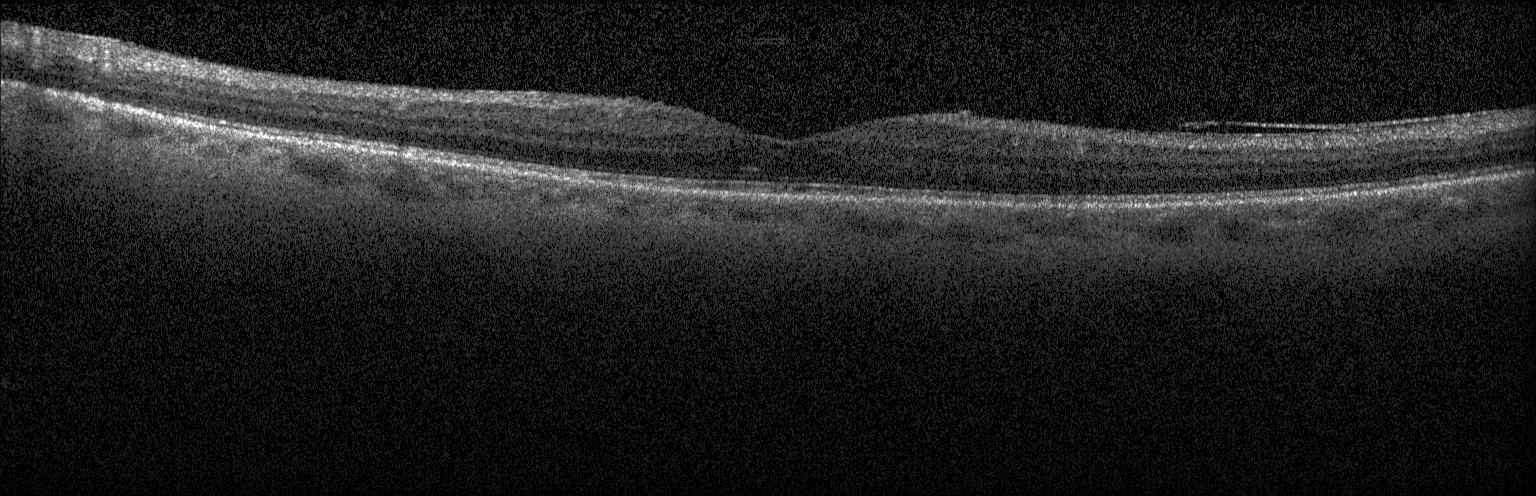
Centered on the fovea · OCT B-scan.
No CNV, DME, or drusen.